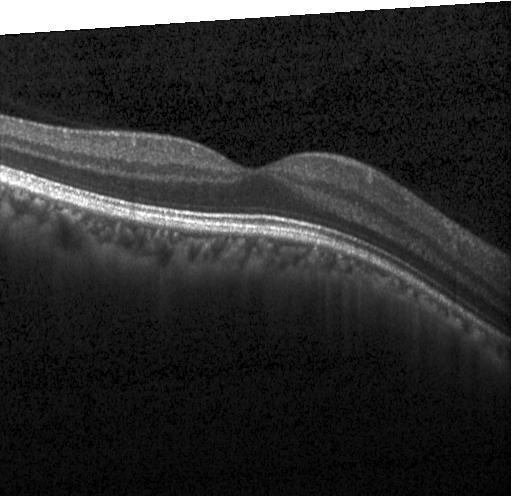 OCT line scan. Finding: no CNV, DME, or drusen.